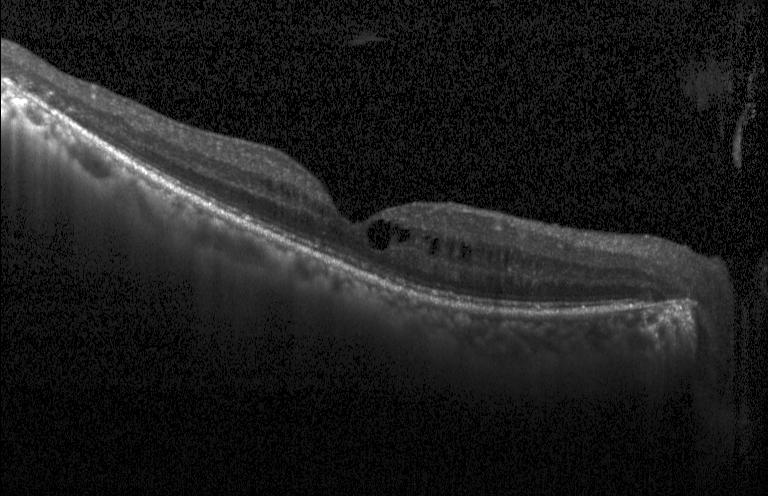

Spectral-domain OCT · through the macula · Heidelberg Spectralis · optical coherence tomography B-scan.
Finding: diabetic macular edema.